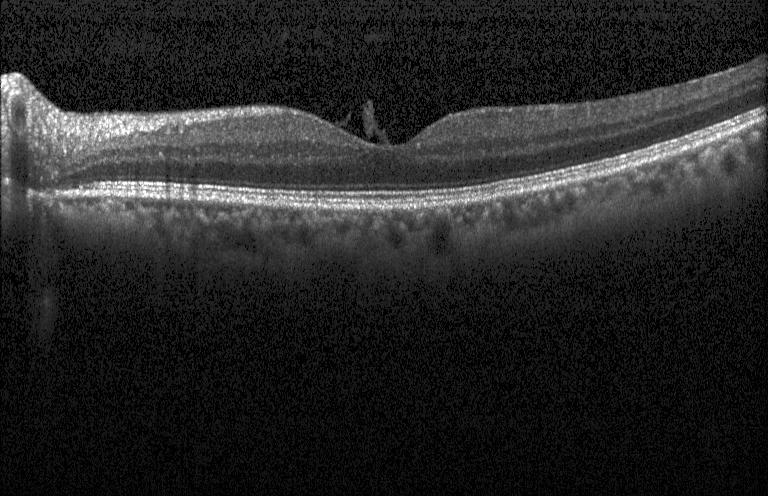

Heidelberg Spectralis. Horizontal scan through the fovea. Retinal OCT B-scan. SD-OCT.
Assessment: neither choroidal neovascularization, diabetic macular edema, nor drusen.